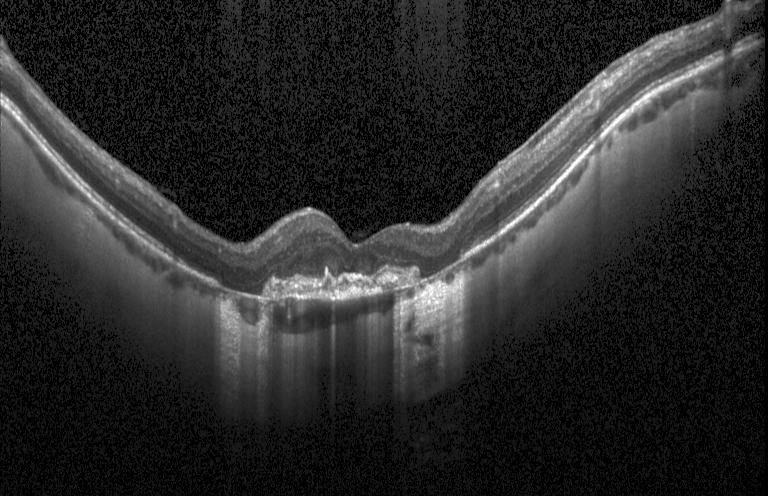 Optical coherence tomography scan
This B-scan demonstrates CNV.